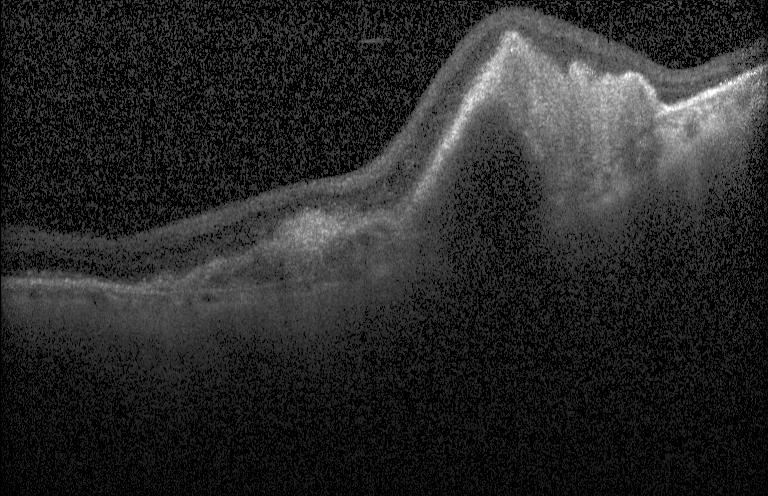
Spectral-domain optical coherence tomography. Acquired on a Heidelberg Spectralis. Optical coherence tomography scan. Fovea-centered — This B-scan demonstrates CNV.